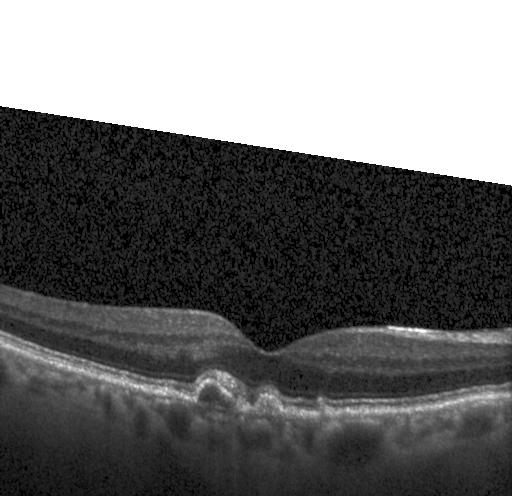
Optical coherence tomography B-scan, centered on the fovea. Diagnosis: a choroidal neovascular membrane.